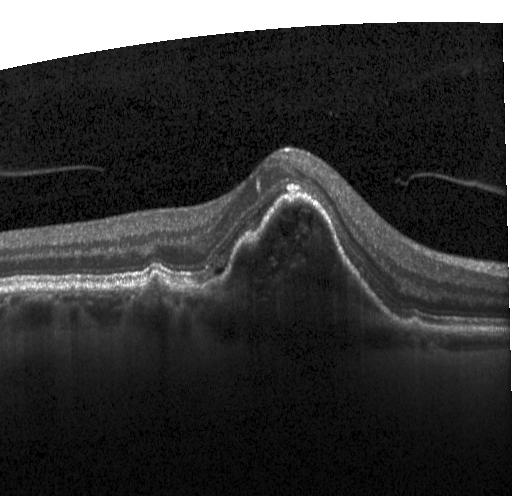 Centered on the fovea · optical coherence tomography B-scan
Macular OCT: choroidal neovascularization (CNV).